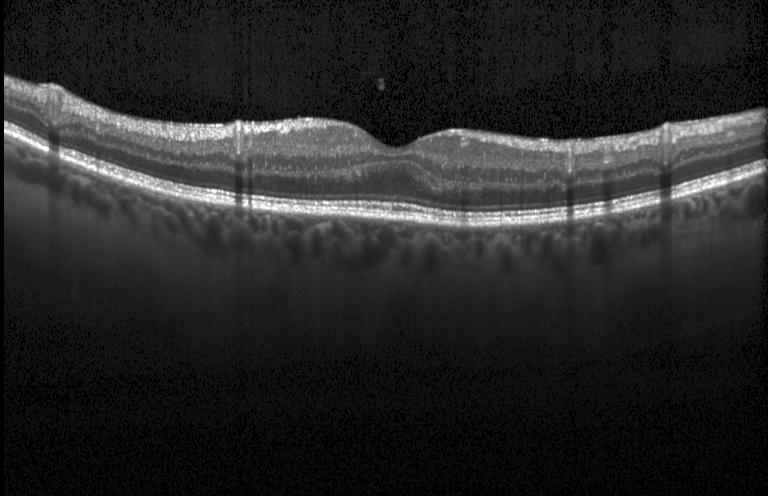
Retinal OCT cross-section.
Diagnosis: no choroidal neovascularization, no diabetic macular edema, and no drusen.